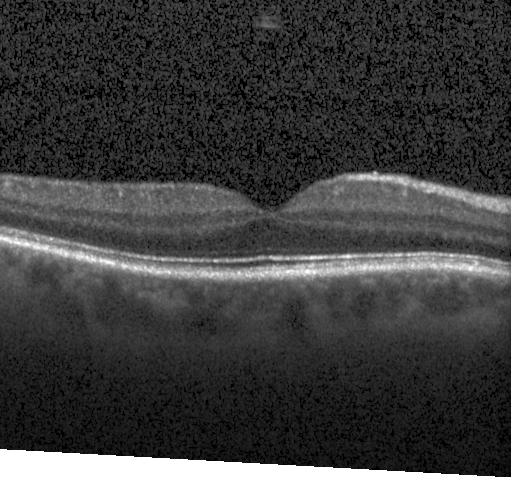
Retinal OCT B-scan — Finding: no choroidal neovascularization, no diabetic macular edema, and no drusen.